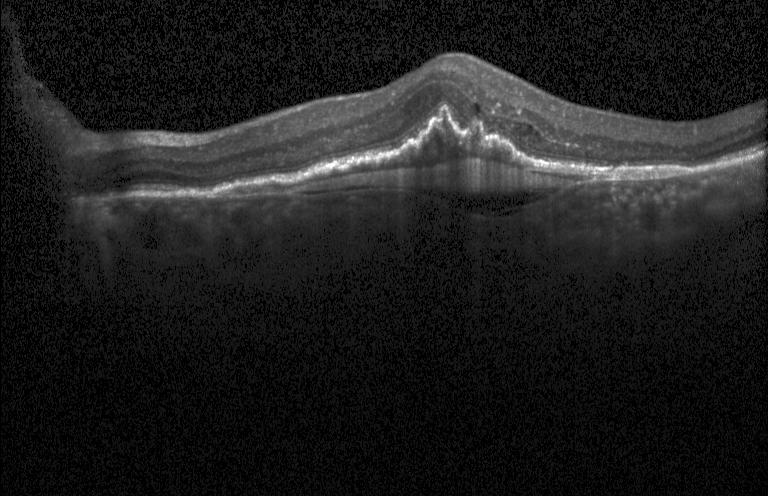 Optical coherence tomography B-scan, acquired on a Heidelberg Spectralis, macular scan
Impression: choroidal neovascularization.